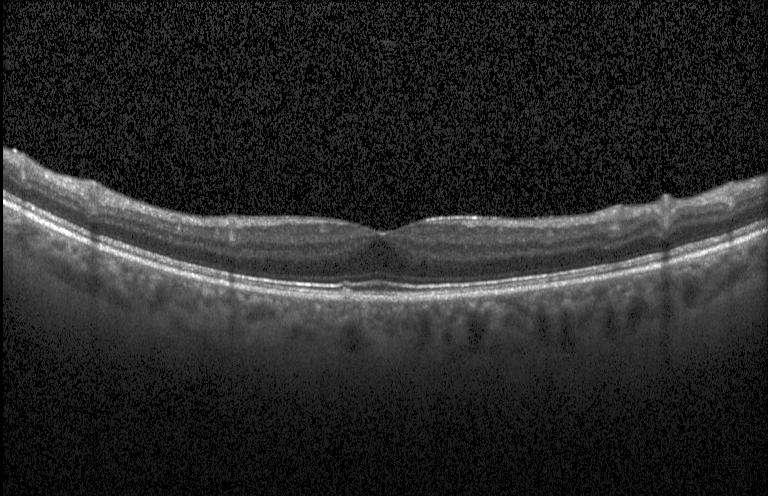 Finding: drusen.